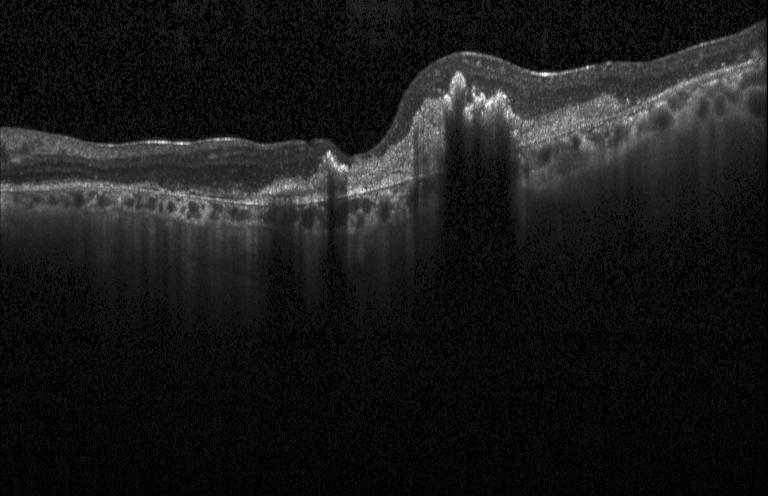

Finding: choroidal neovascularization (CNV).